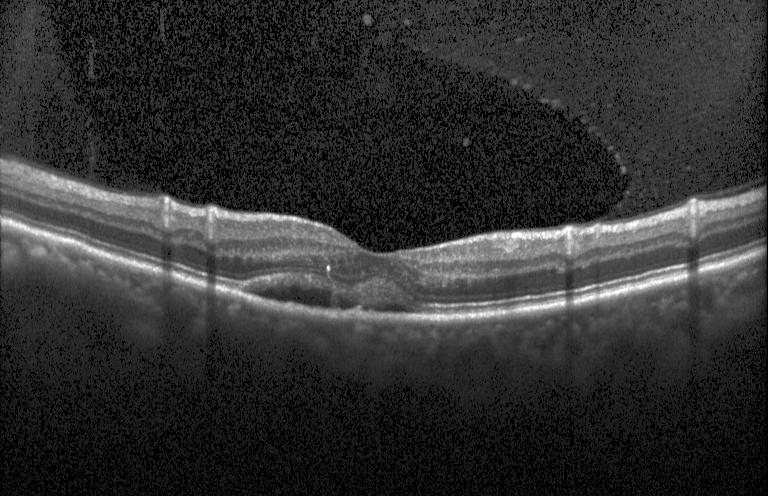 OCT line scan. OCT finding: a choroidal neovascular membrane.